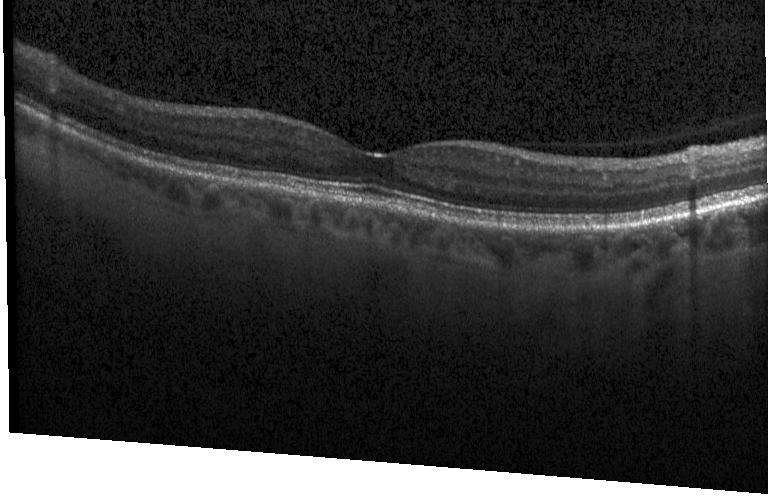
Dx: no CNV, no DME, and no drusen.